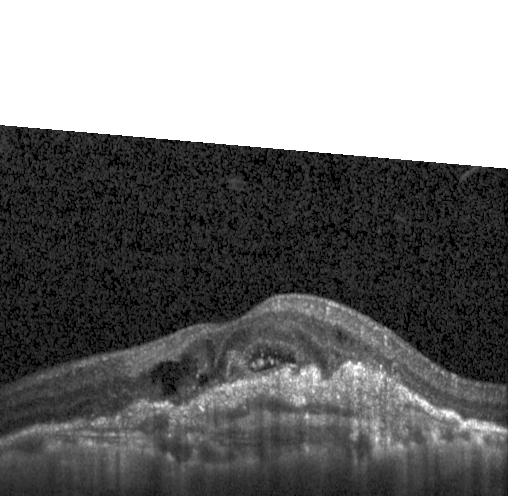

OCT B-scan showing a choroidal neovascular membrane.